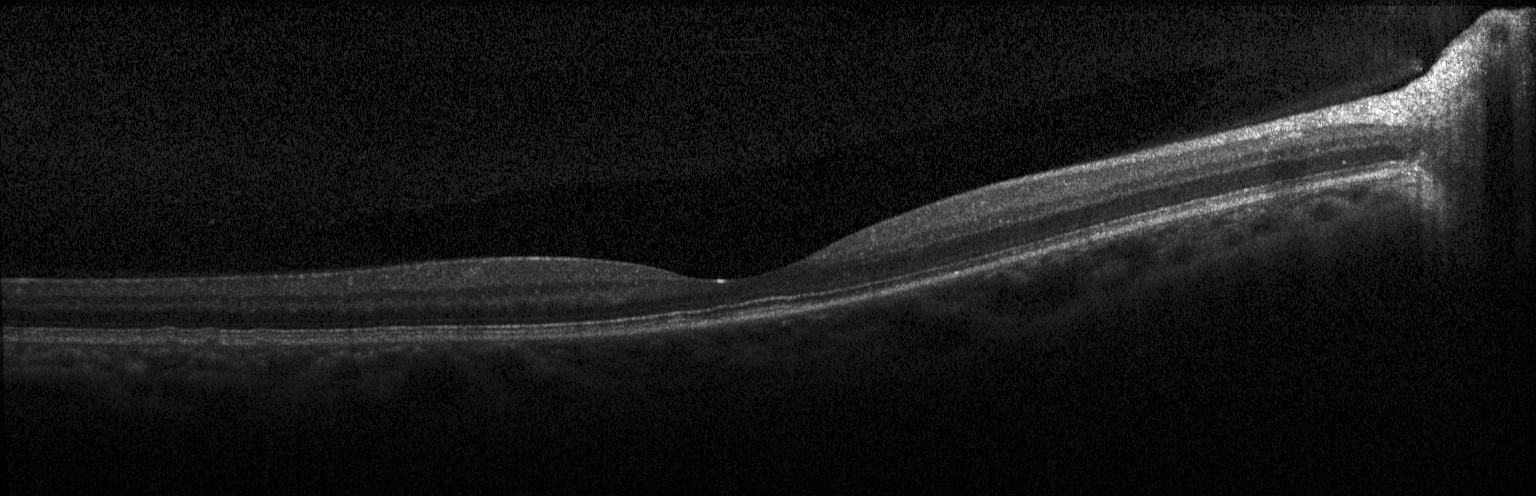

Fovea-centered · retinal OCT cross-section
Finding: no CNV, no DME, and no drusen.